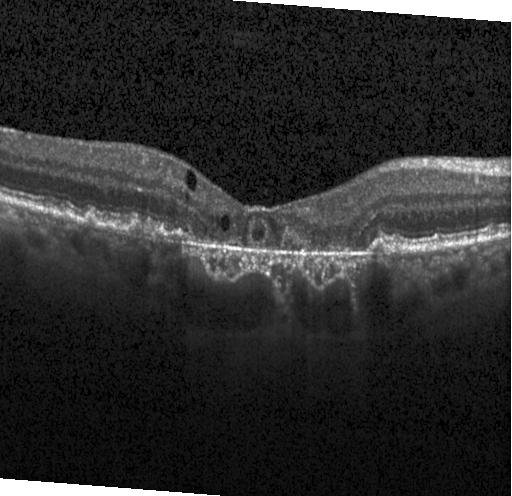
OCT B-scan. The scan shows choroidal neovascularization.